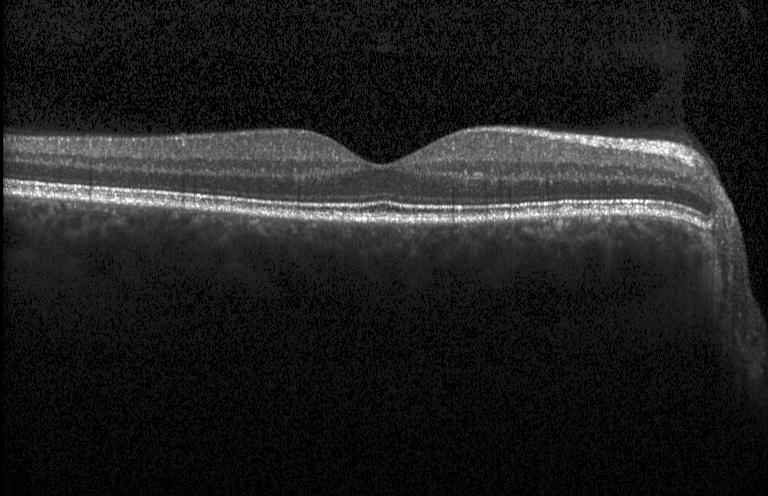
Optical coherence tomography scan.
OCT finding: no choroidal neovascularization, no diabetic macular edema, and no drusen.